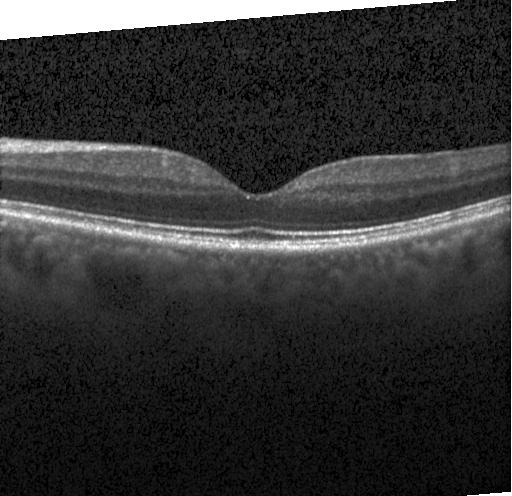 Optical coherence tomography B-scan. Impression: no evidence of choroidal neovascularization, diabetic macular edema, or drusen.